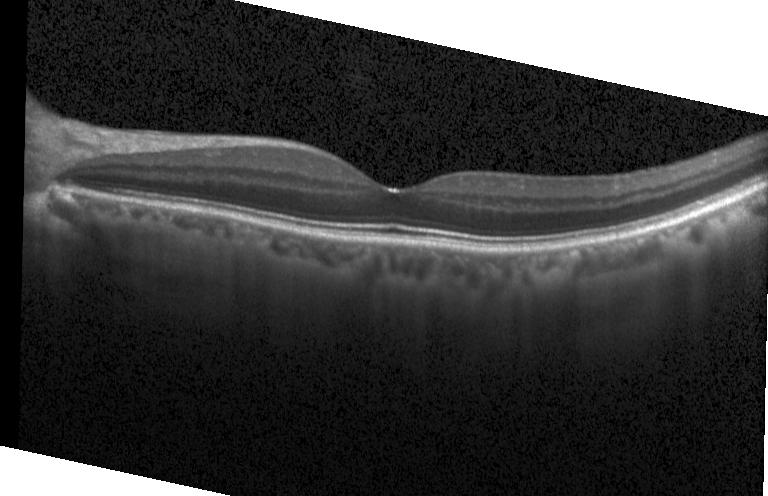
Retinal OCT B-scan · SD-OCT — Macular OCT: no CNV, no DME, and no drusen.